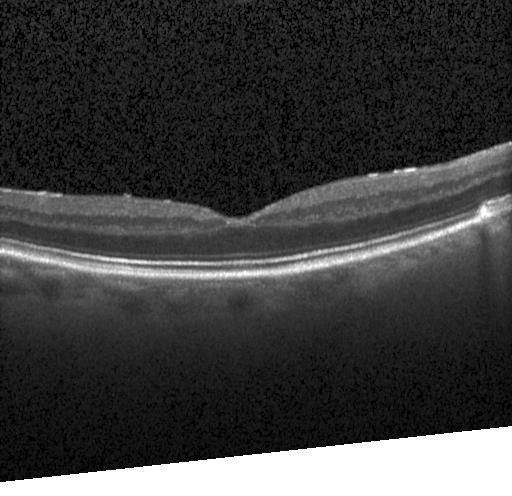 Horizontal scan through the fovea · optical coherence tomography scan — Diagnosis: neither CNV, DME, nor drusen.